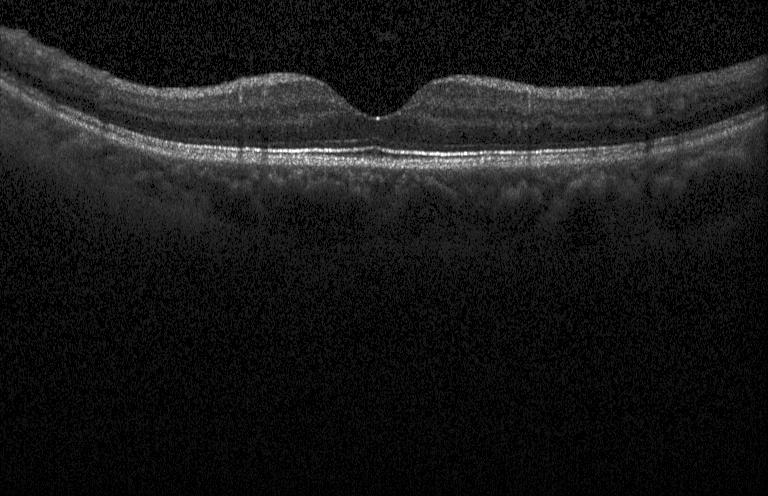 OCT scan showing neither choroidal neovascularization, diabetic macular edema, nor drusen.